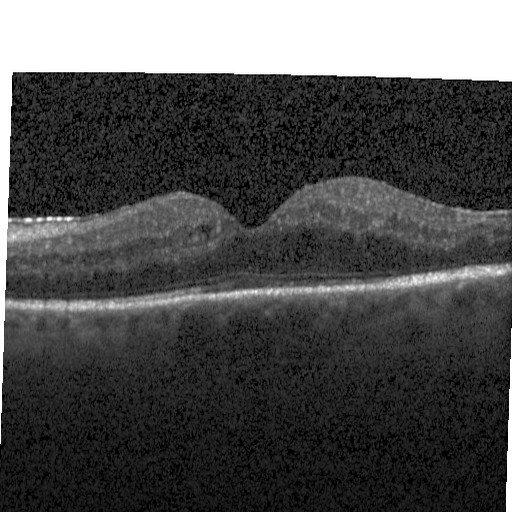
DME.